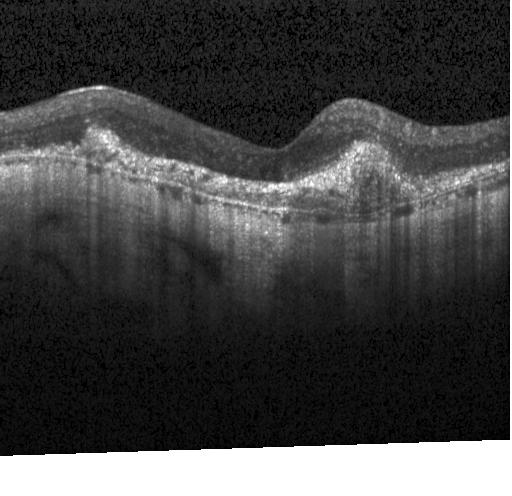
OCT scan showing choroidal neovascularization (CNV).